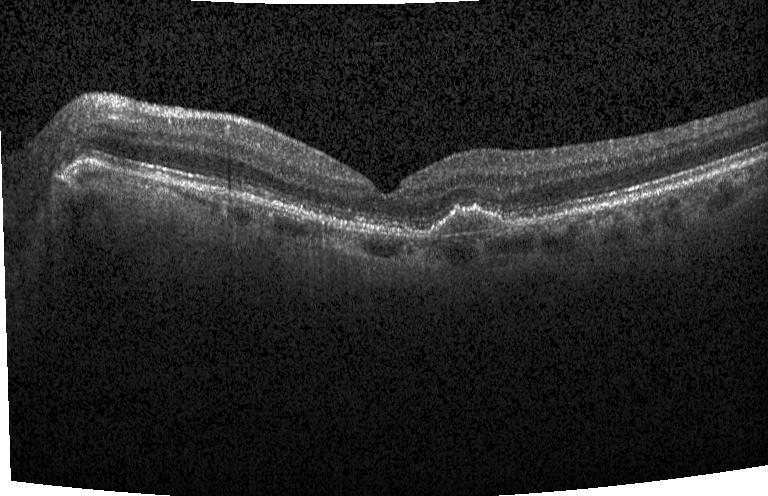

Horizontal scan through the fovea; retinal OCT cross-section
Impression: a choroidal neovascular membrane.